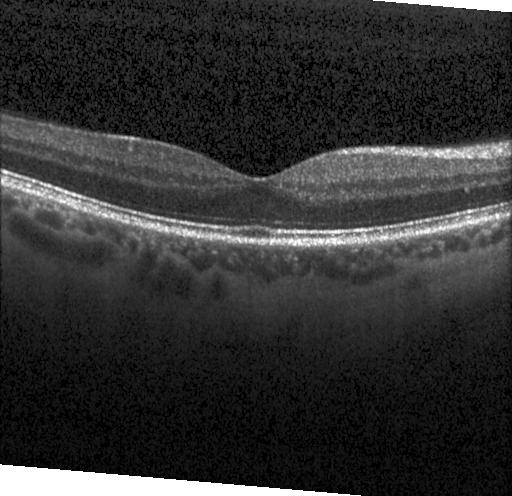
Finding: neither CNV, DME, nor drusen.